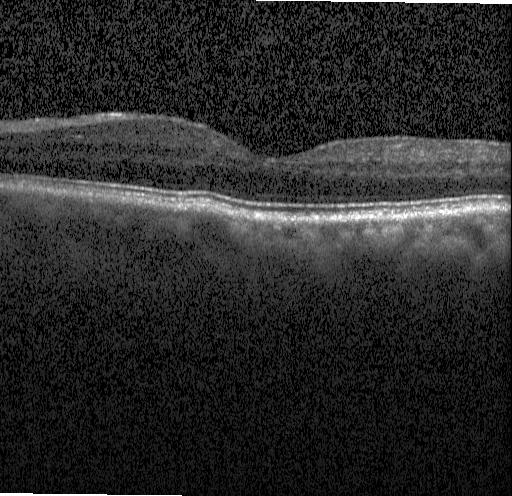

Centered on the fovea · optical coherence tomography scan · instrument: Heidelberg Spectralis. Diagnosis: no choroidal neovascularization, diabetic macular edema, or drusen.